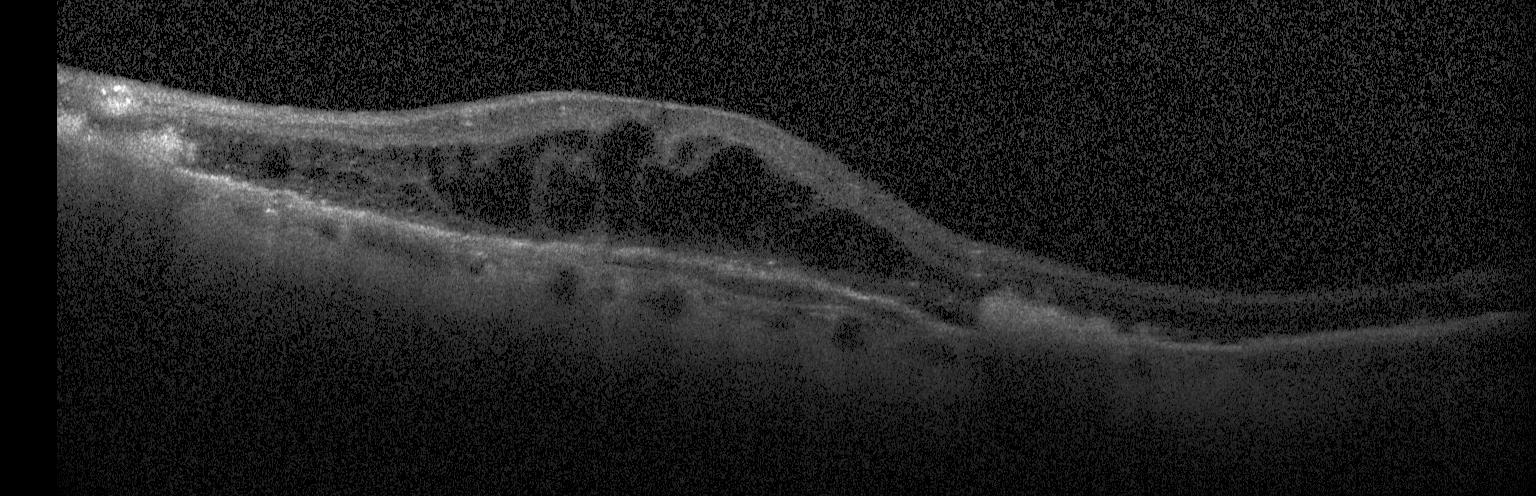
This B-scan demonstrates a choroidal neovascular membrane.